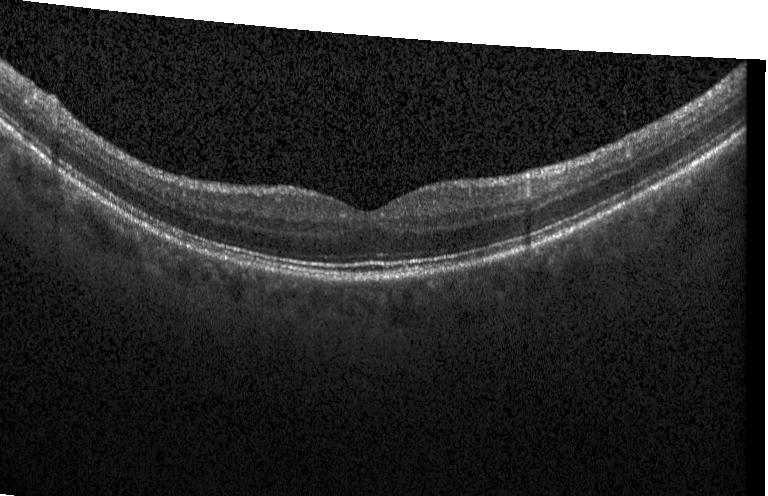

Fovea-centered. OCT B-scan. SD-OCT. Acquired on a Heidelberg Spectralis. The scan shows no CNV, no DME, and no drusen.